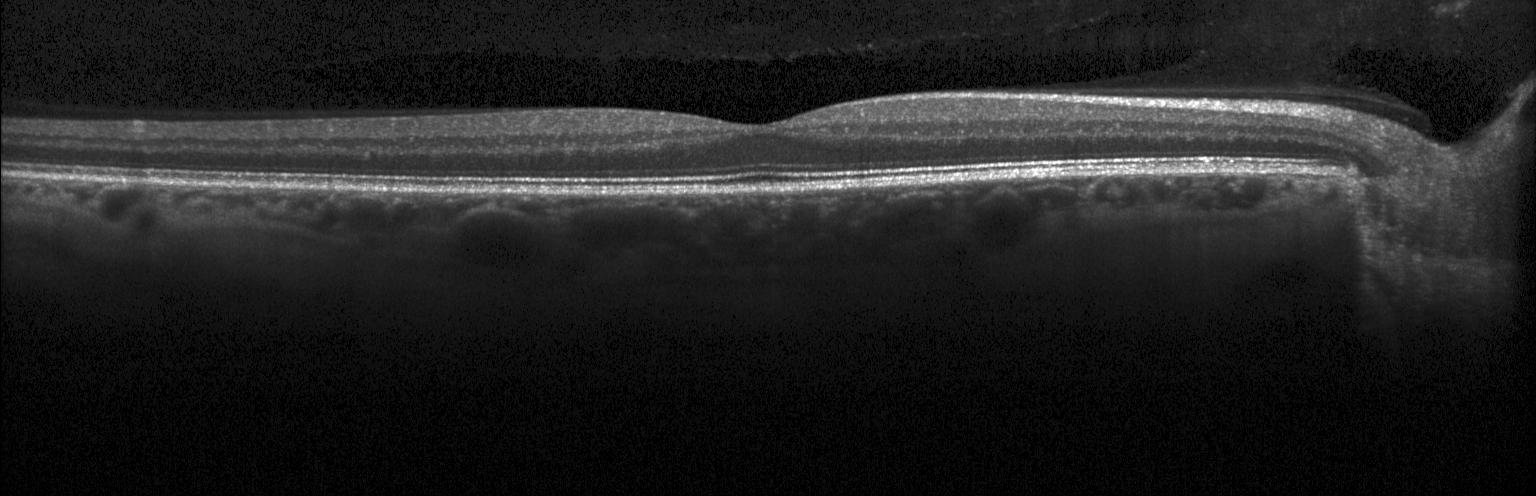
Impression: no CNV, no DME, and no drusen.